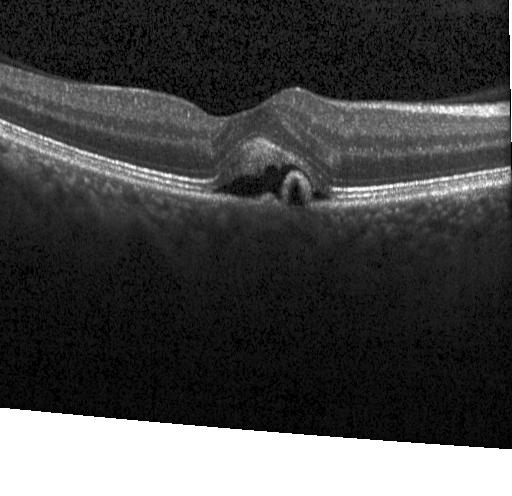

Spectral-domain OCT. Retinal OCT B-scan. Heidelberg Spectralis OCT system. The scan shows CNV.